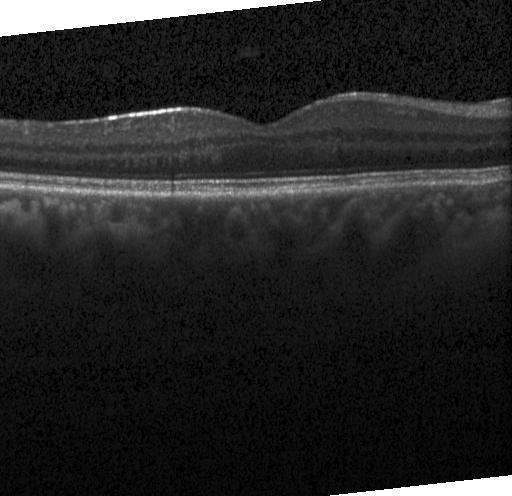
SD-OCT; Heidelberg Spectralis; OCT B-scan; centered on the fovea. This B-scan demonstrates no evidence of choroidal neovascularization, diabetic macular edema, or drusen.